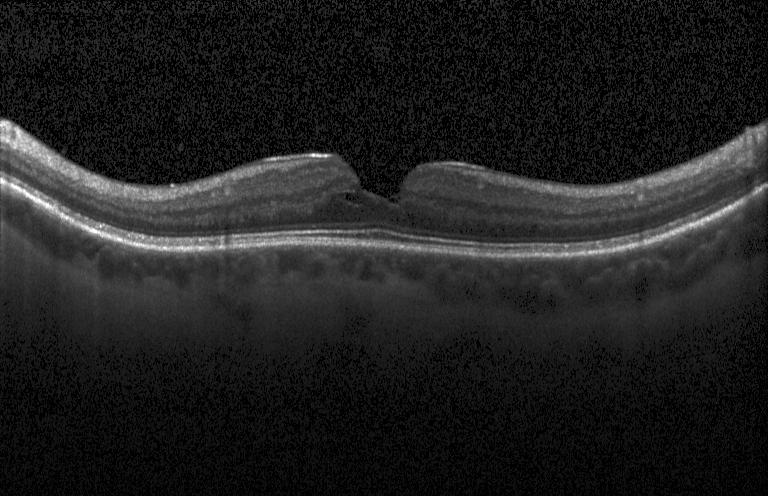
OCT B-scan; through the macula; acquired on a Heidelberg Spectralis; spectral-domain optical coherence tomography
Assessment: diabetic macular edema.